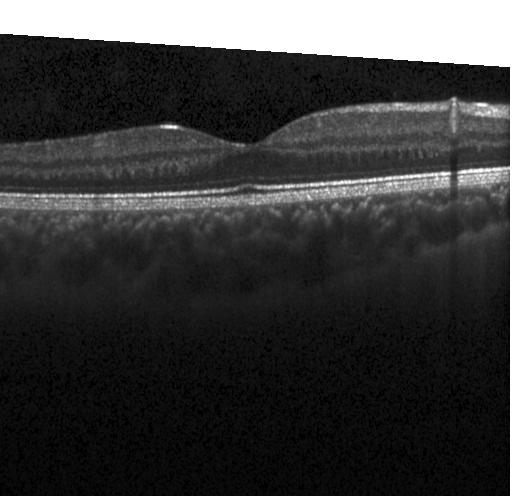
No choroidal neovascularization, diabetic macular edema, or drusen.